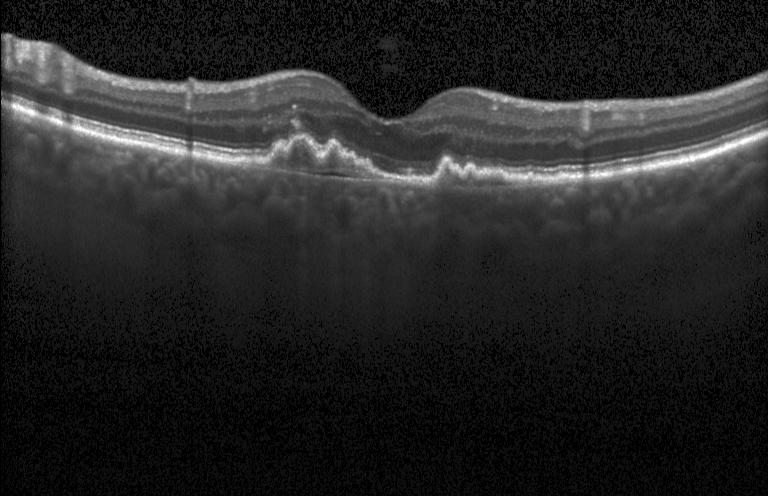

OCT scan showing a choroidal neovascular membrane.